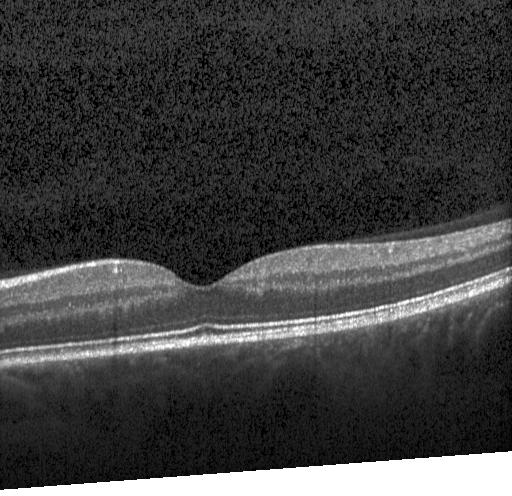 Retinal OCT B-scan. Through the macula — Diagnosis: neither CNV, DME, nor drusen.